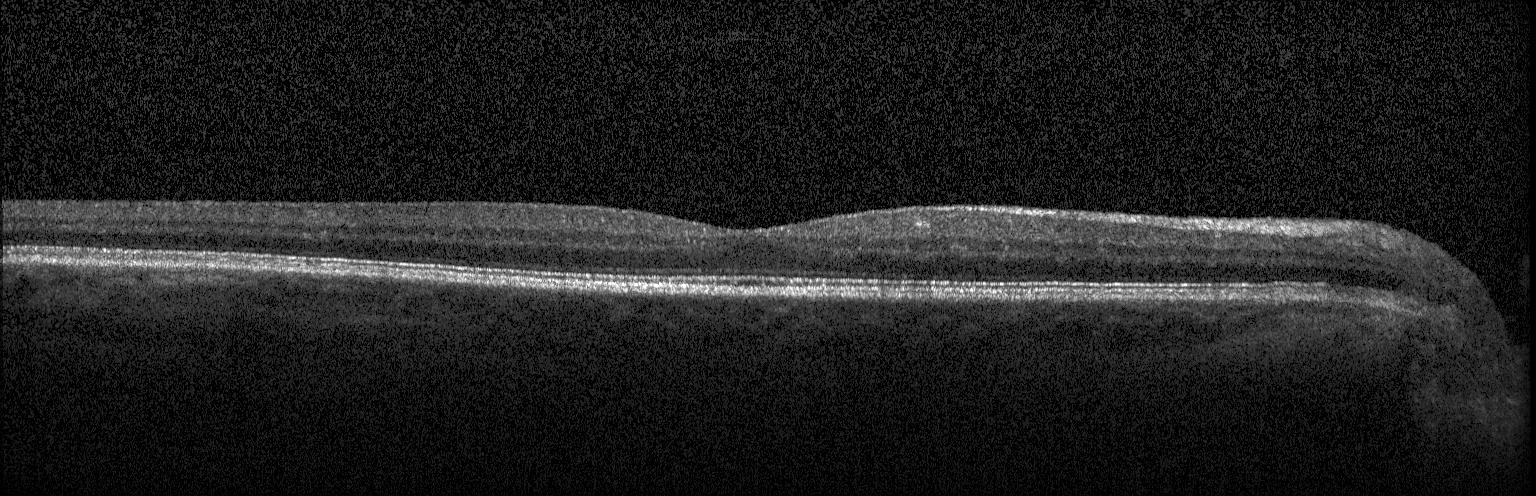

Retinal OCT cross-section — Assessment: no evidence of choroidal neovascularization, diabetic macular edema, or drusen.